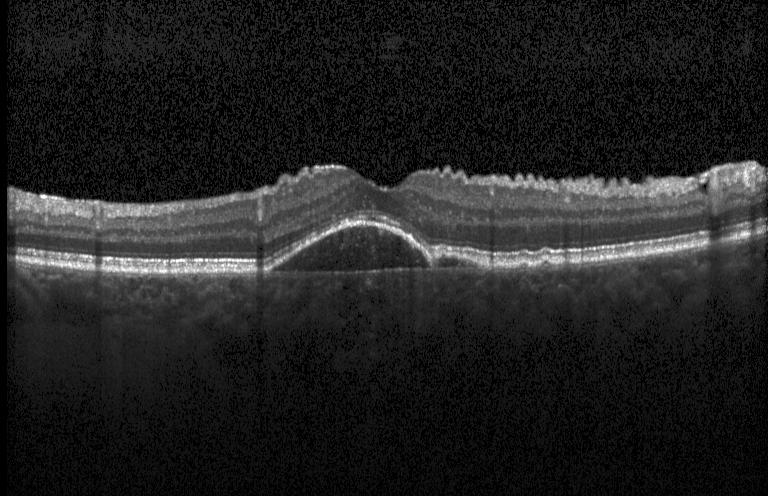
Spectral-domain OCT B-scan: choroidal neovascularization.